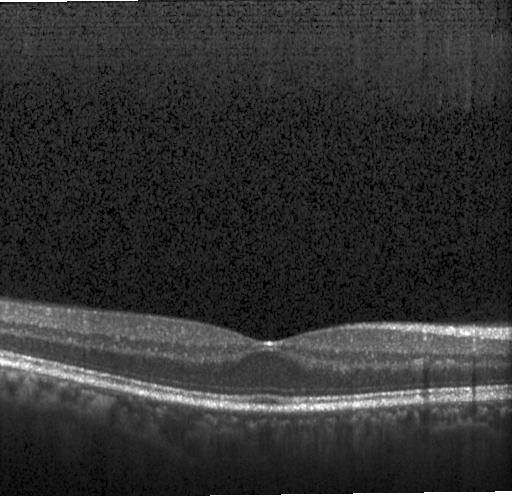

Macular OCT demonstrating no evidence of choroidal neovascularization, diabetic macular edema, or drusen.